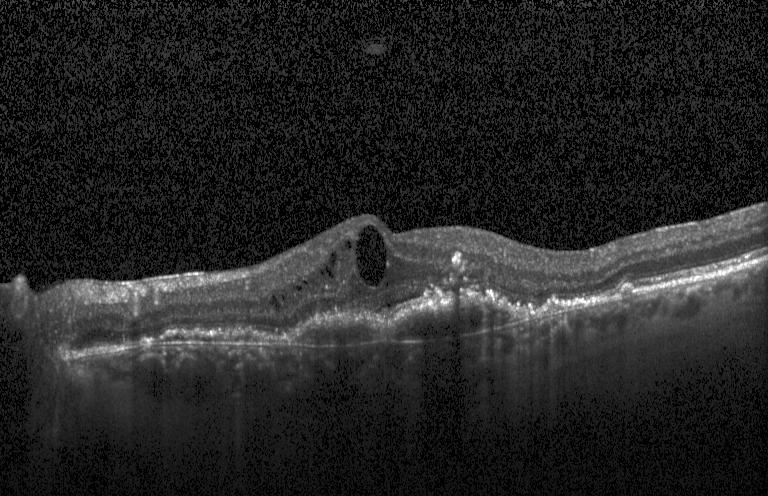 OCT line scan
CNV.